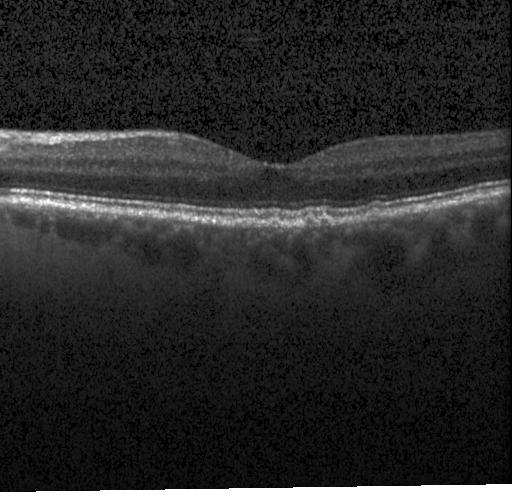
Retinal OCT cross-section; acquired on a Heidelberg Spectralis
OCT finding: multiple drusen.